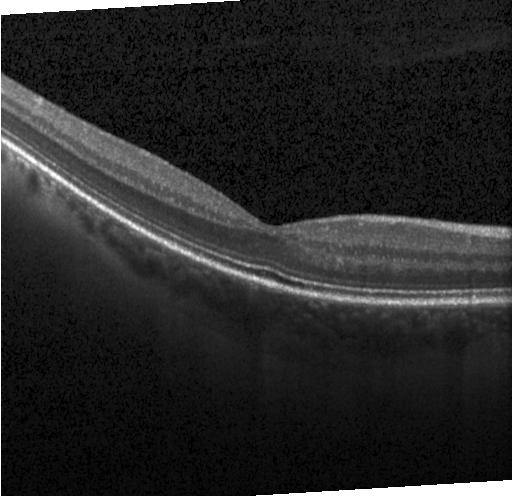

OCT B-scan showing no CNV, DME, or drusen.